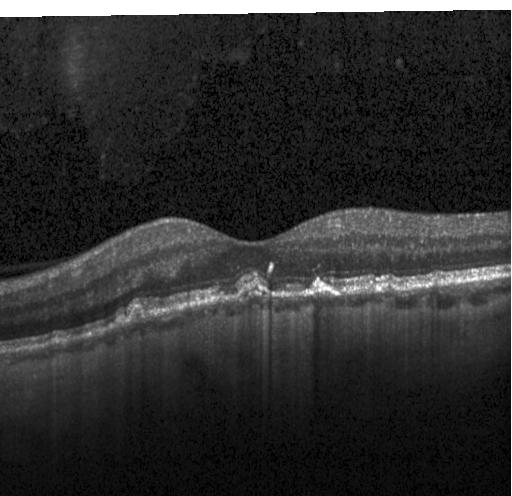
Diagnosis: a choroidal neovascular membrane.